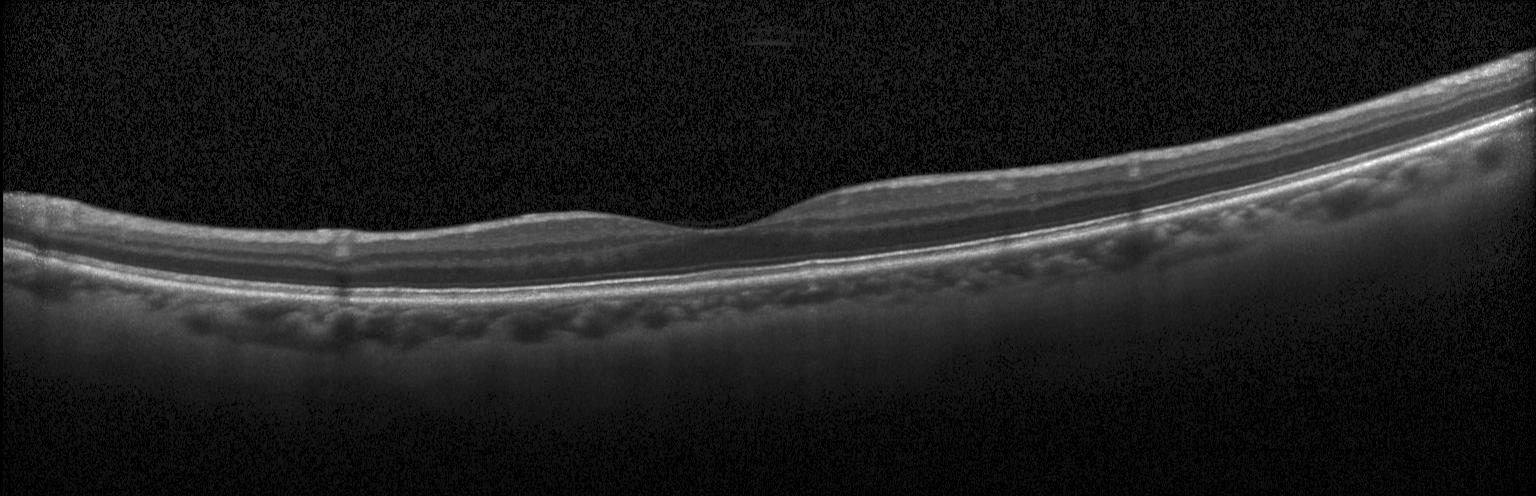 The scan shows no choroidal neovascularization, no diabetic macular edema, and no drusen.